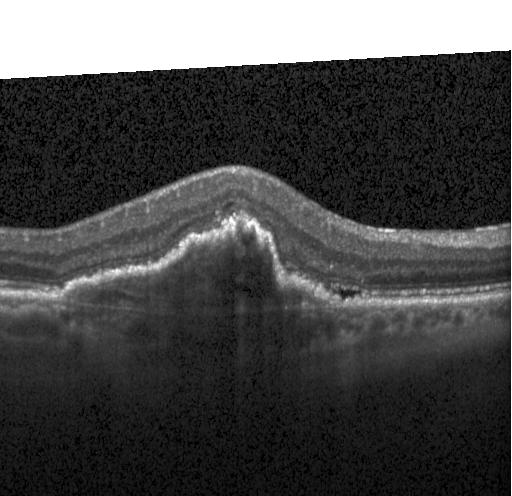
OCT B-scan showing a choroidal neovascular membrane.